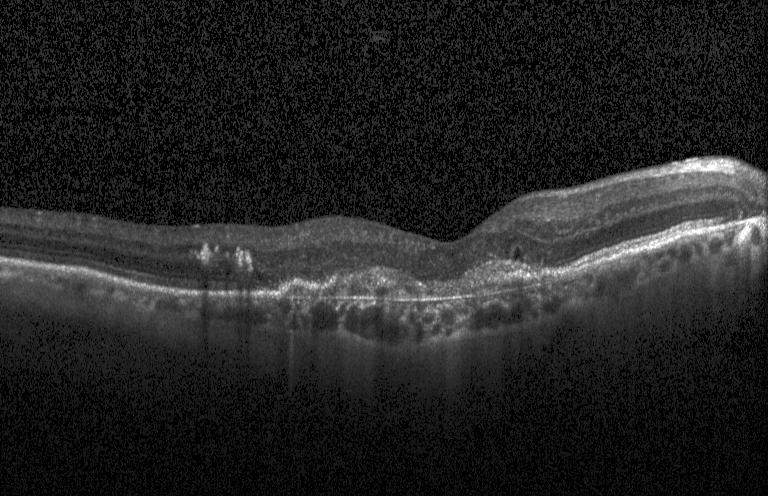

Choroidal neovascularization.